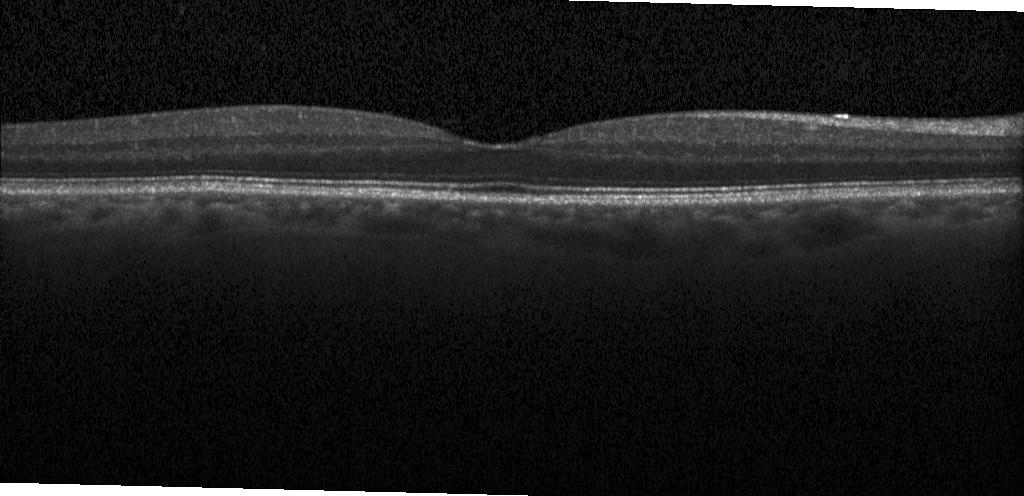 OCT B-scan; fovea-centered; Heidelberg Spectralis; SD-OCT. Diagnosis: no choroidal neovascularization, no diabetic macular edema, and no drusen.